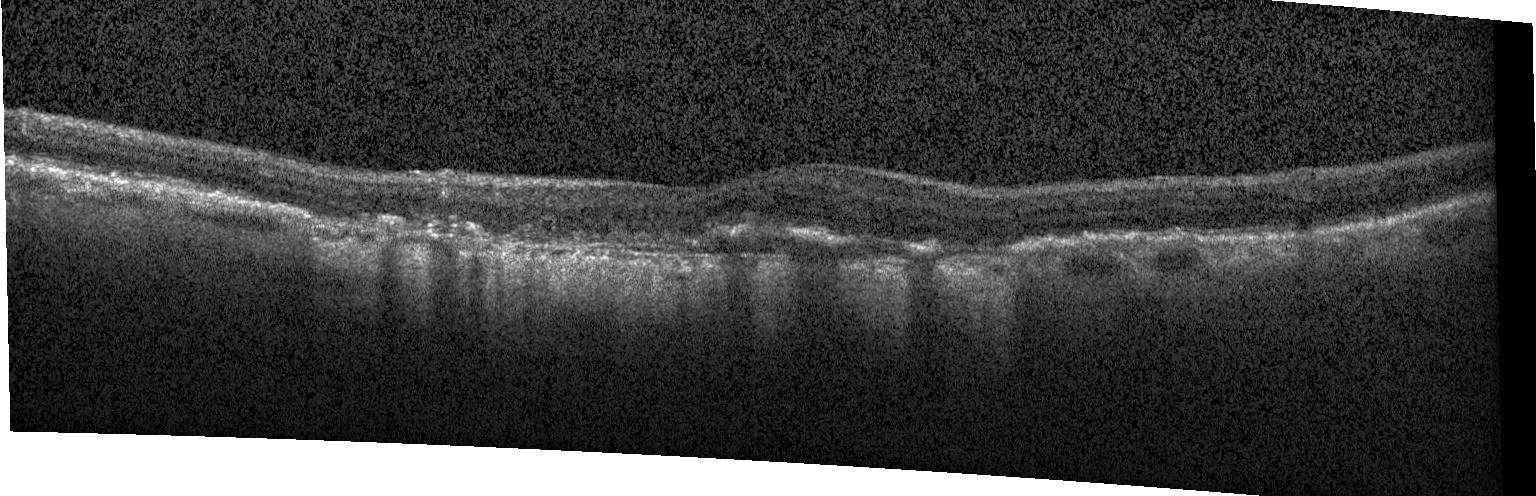

Optical coherence tomography scan.
OCT finding: a choroidal neovascular membrane.